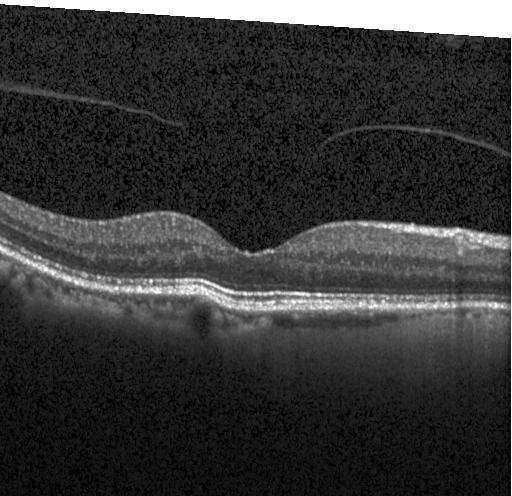 The scan shows no CNV, DME, or drusen.